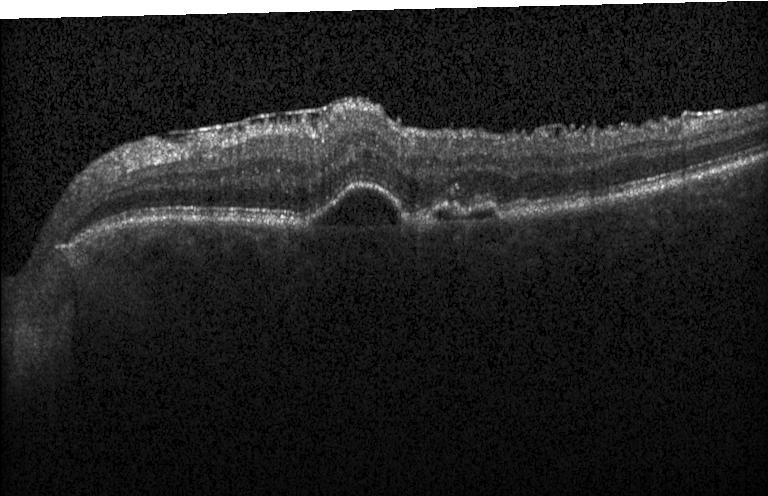

Retinal OCT B-scan.
Choroidal neovascularization (CNV).